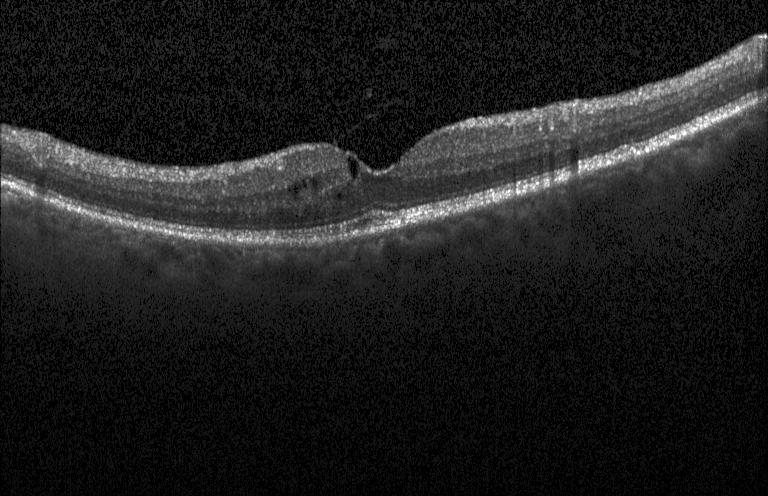 Heidelberg Spectralis OCT system; spectral-domain optical coherence tomography; macular scan; optical coherence tomography scan
Finding: DME.